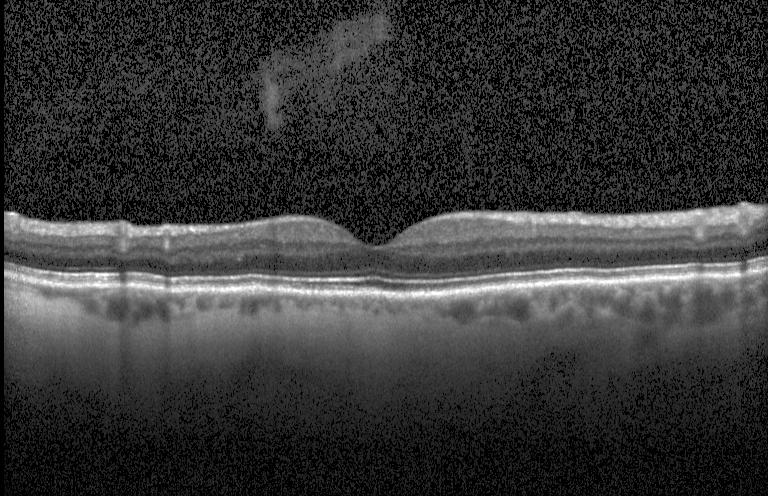

Finding: no choroidal neovascularization, diabetic macular edema, or drusen.